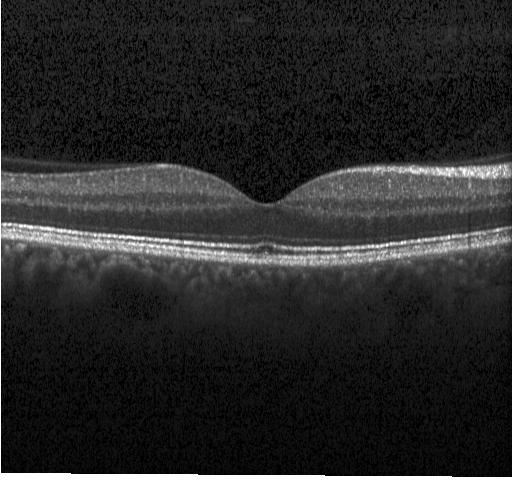

Impression: no choroidal neovascularization, diabetic macular edema, or drusen.